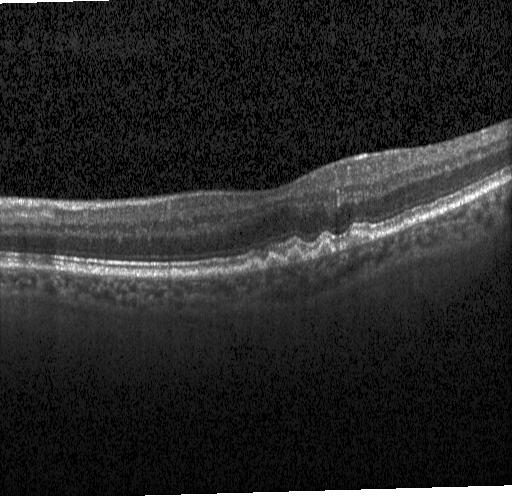
Optical coherence tomography scan — Macular OCT: drusen.